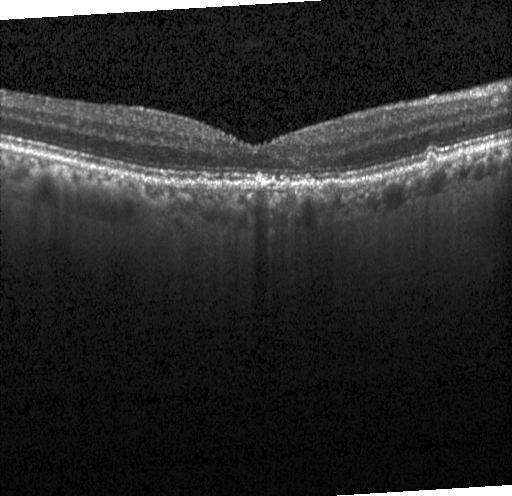
Retinal OCT B-scan. Heidelberg Spectralis. Centered on the fovea — Assessment: drusen.